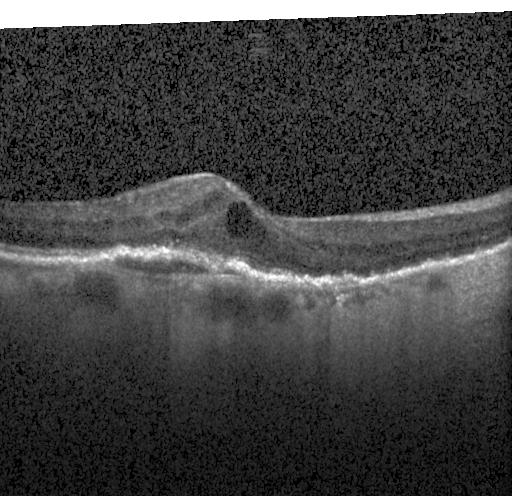

Retinal OCT B-scan, horizontal scan through the fovea, Heidelberg Spectralis OCT system. Choroidal neovascularization.